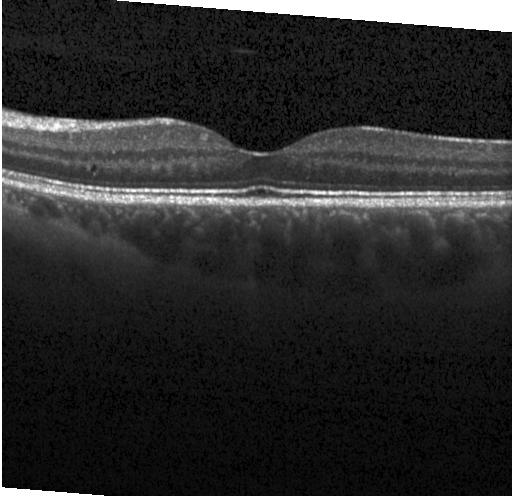

Spectral-domain OCT B-scan: no choroidal neovascularization, no diabetic macular edema, and no drusen.